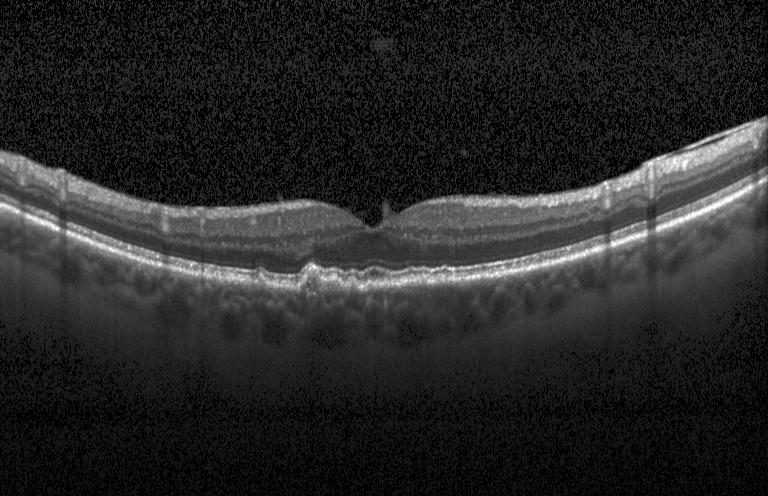

Instrument: Heidelberg Spectralis. Optical coherence tomography scan. Fovea-centered. Dx: multiple drusen.